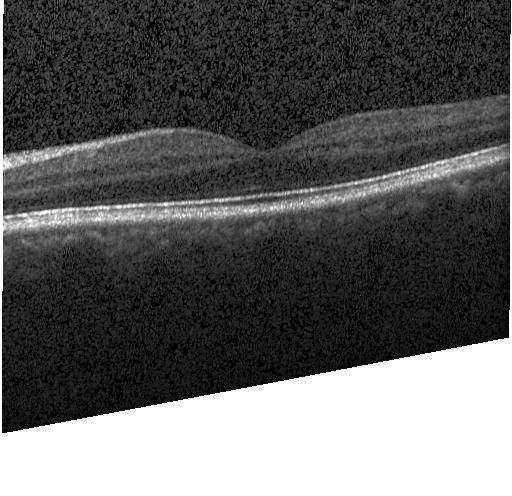

Retinal OCT cross-section, spectral-domain optical coherence tomography
Macular OCT: neither choroidal neovascularization, diabetic macular edema, nor drusen.